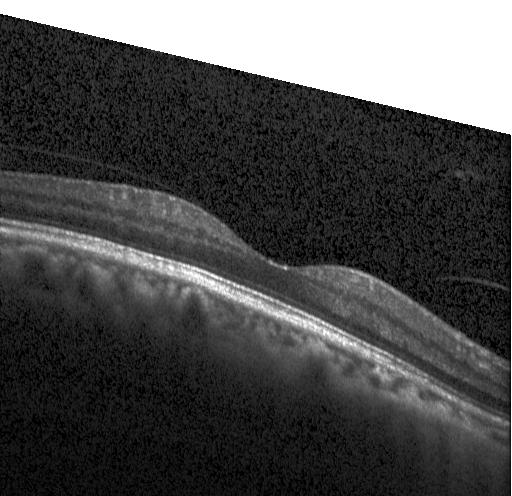
Optical coherence tomography scan. Instrument: Heidelberg Spectralis. Macular OCT: no CNV, DME, or drusen.